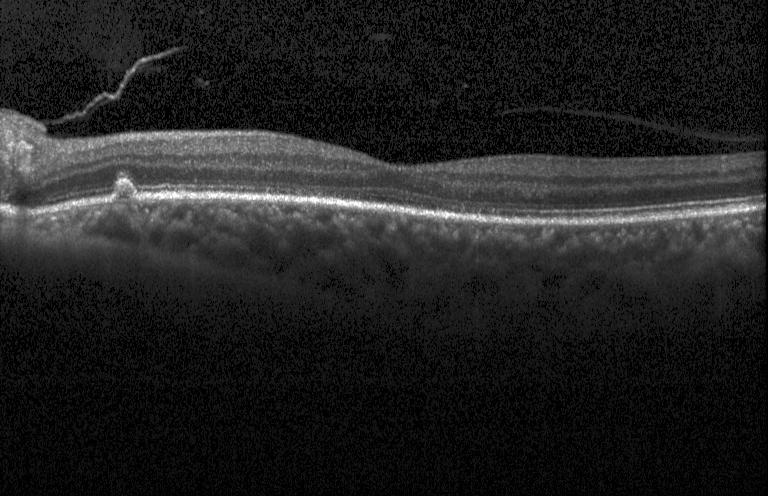

Finding: drusen.